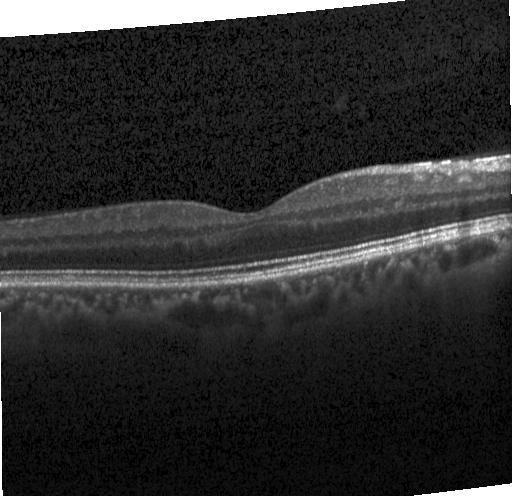 Macular OCT: neither choroidal neovascularization, diabetic macular edema, nor drusen.